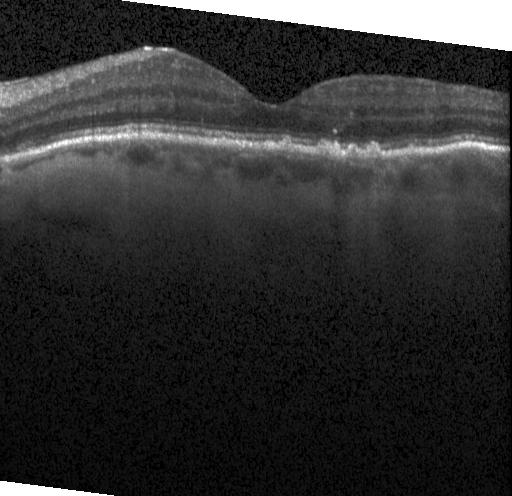 Retinal OCT cross-section
This B-scan demonstrates drusen.